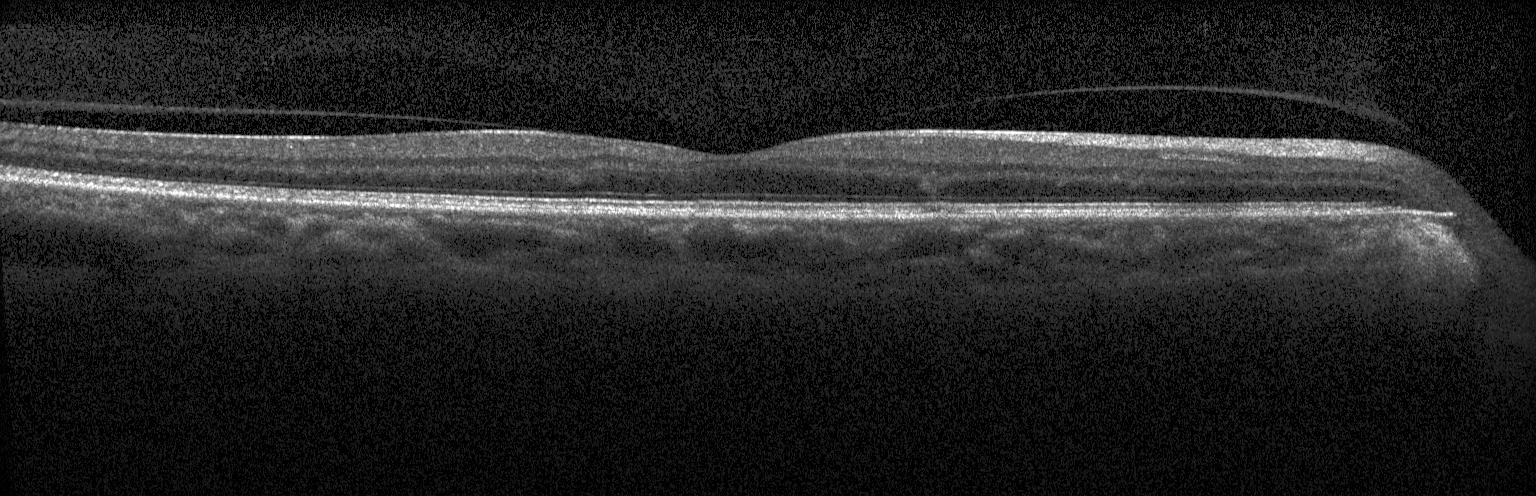
Spectral-domain optical coherence tomography; optical coherence tomography scan.
OCT finding: no CNV, no DME, and no drusen.